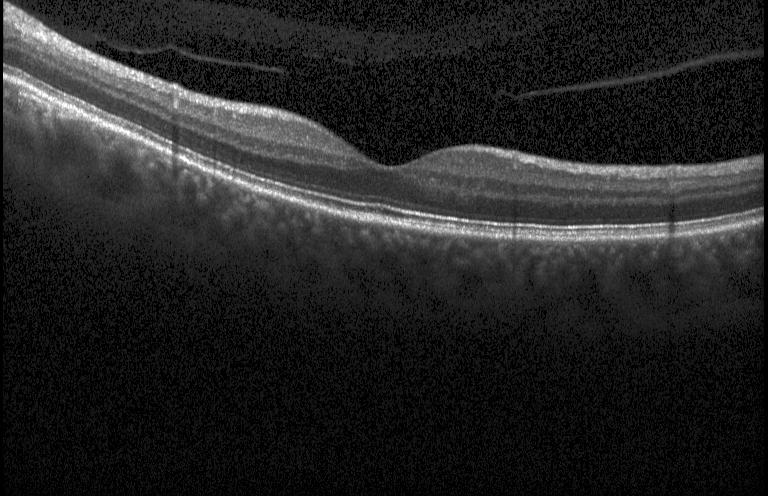 OCT B-scan. Finding: neither CNV, DME, nor drusen.